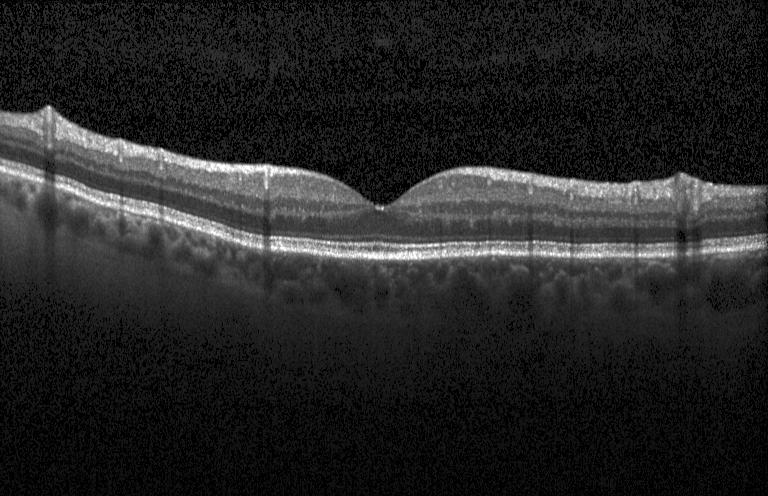 Macular OCT demonstrating neither choroidal neovascularization, diabetic macular edema, nor drusen.